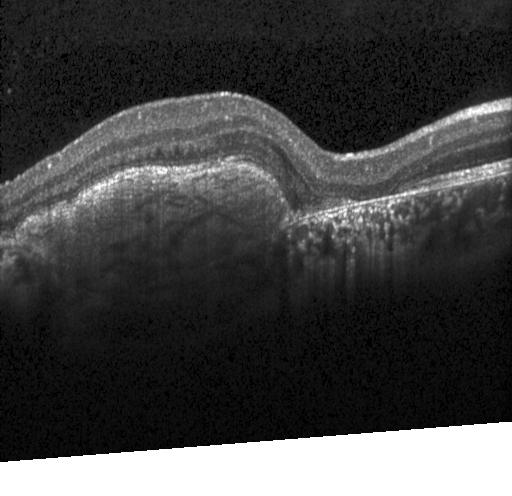
A choroidal neovascular membrane.